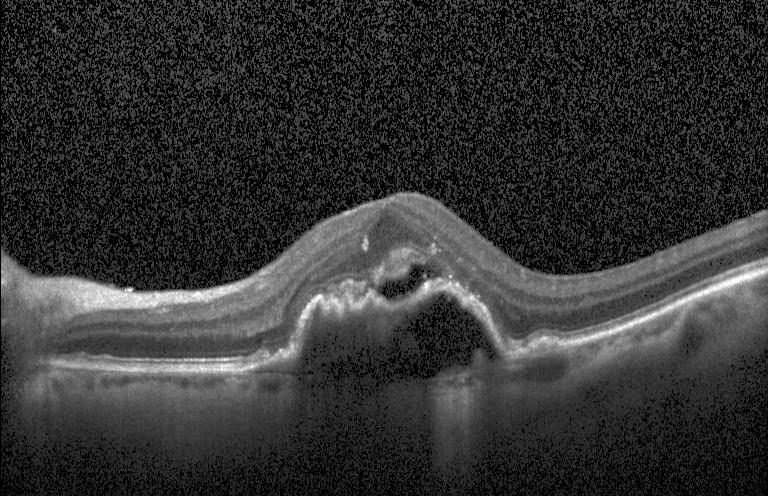 Finding: a choroidal neovascular membrane.